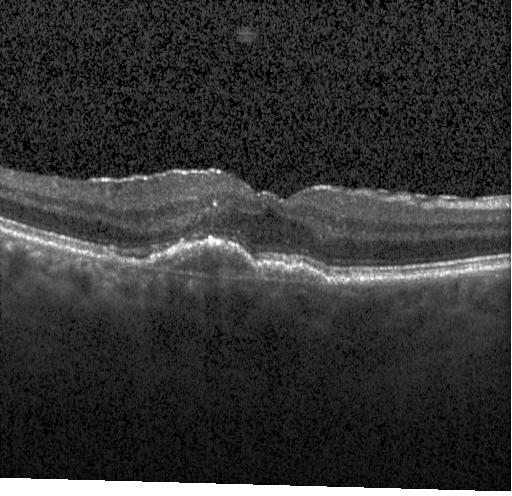
Retinal OCT cross-section
Impression: a choroidal neovascular membrane.